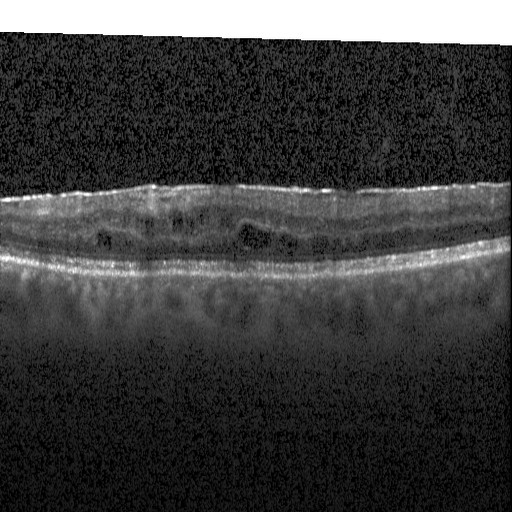

Retinal OCT B-scan; macular scan
Finding: diabetic macular edema (DME).